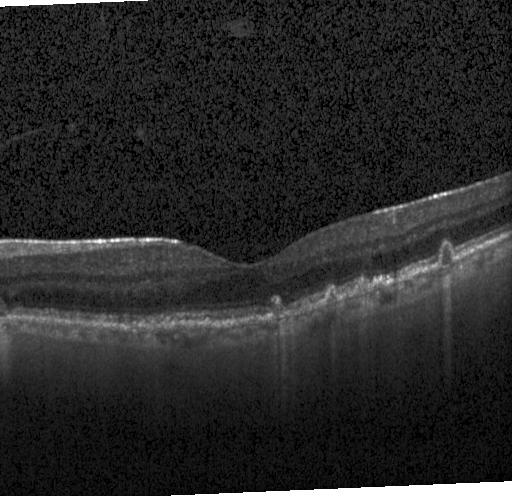
SD-OCT, OCT B-scan. This B-scan demonstrates multiple drusen.